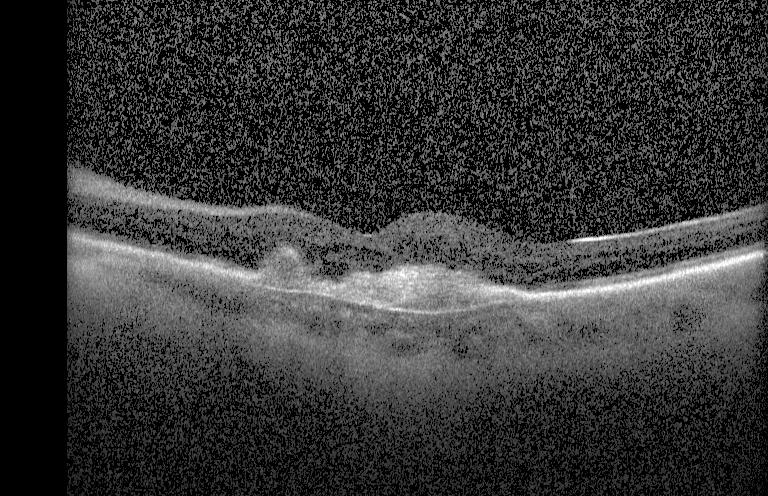

Fovea-centered · OCT B-scan · instrument: Heidelberg Spectralis
Assessment: CNV.